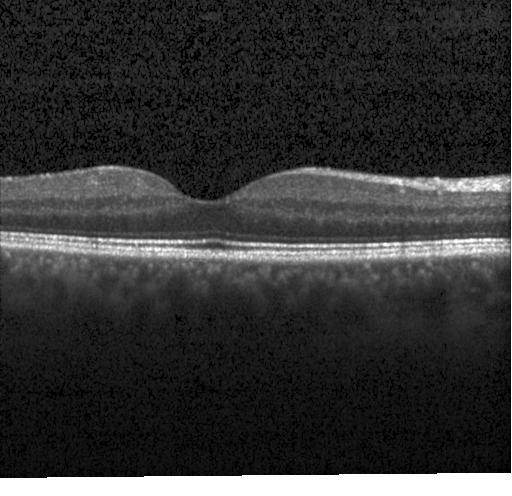 Diagnosis: no choroidal neovascularization, diabetic macular edema, or drusen.